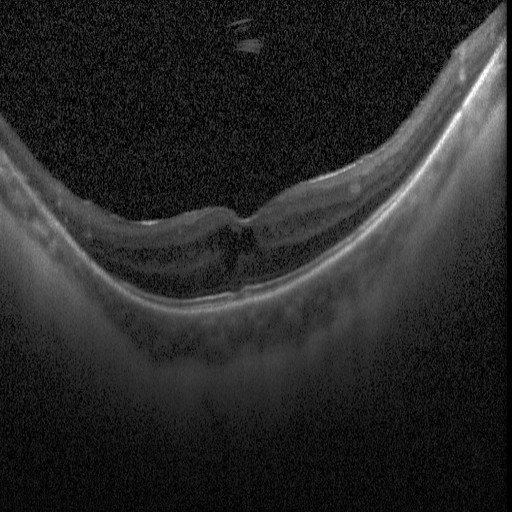

SD-OCT, fovea-centered, OCT line scan, Heidelberg Spectralis OCT system. Macular OCT: diabetic macular edema (DME).